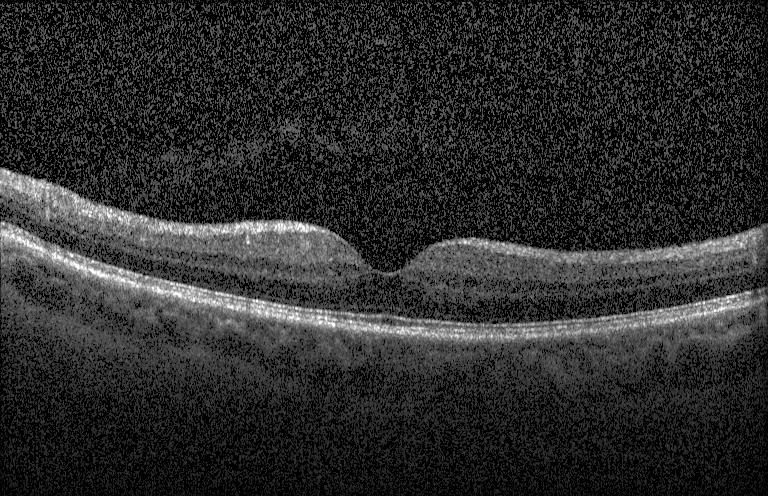
Optical coherence tomography scan · Heidelberg Spectralis OCT system.
Diagnosis: no CNV, DME, or drusen.